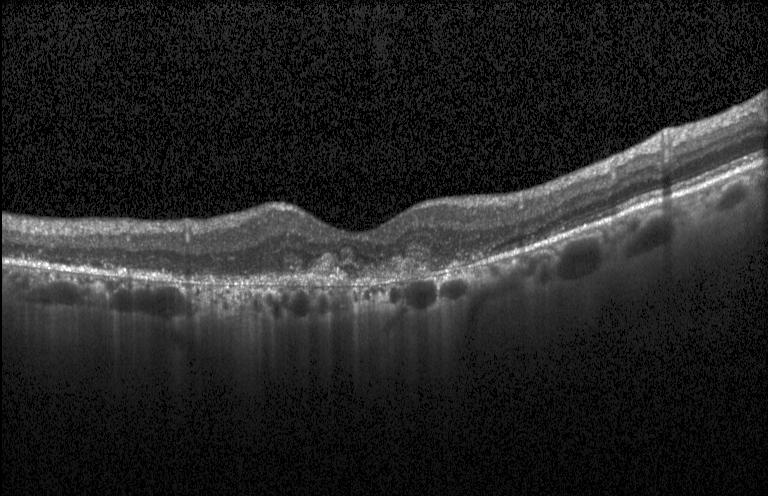 Optical coherence tomography B-scan; horizontal scan through the fovea; spectral-domain OCT — Impression: choroidal neovascularization.